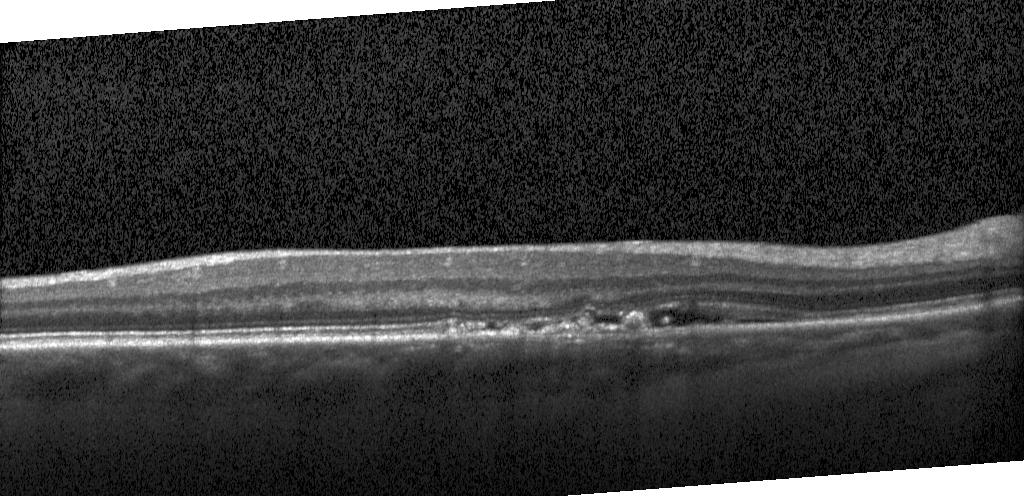 Macular OCT: choroidal neovascularization.